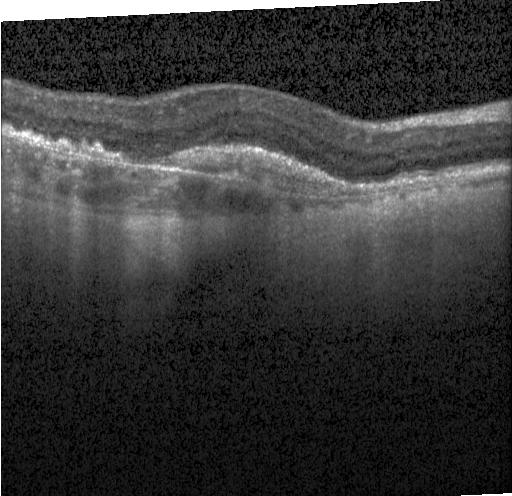 Diagnosis: a choroidal neovascular membrane.